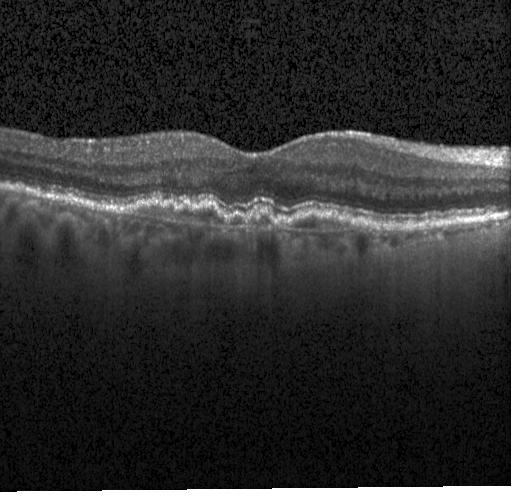

Retinal OCT cross-section showing a choroidal neovascular membrane.